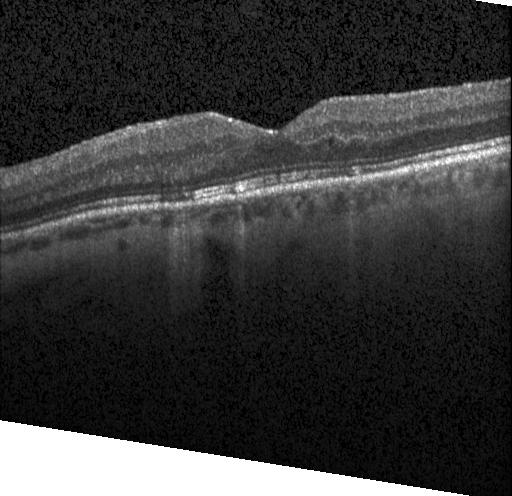
OCT finding: neither choroidal neovascularization, diabetic macular edema, nor drusen.